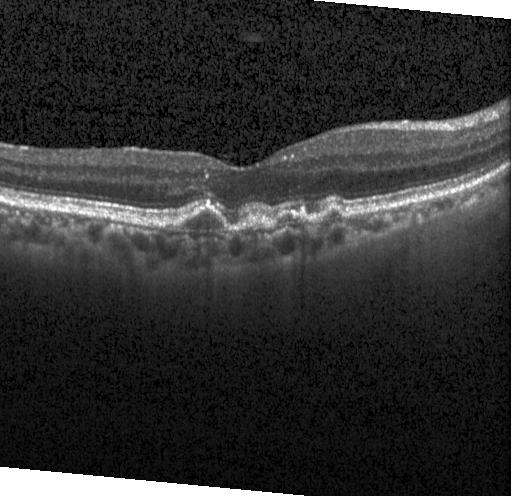
Retinal OCT B-scan. Diagnosis: CNV.